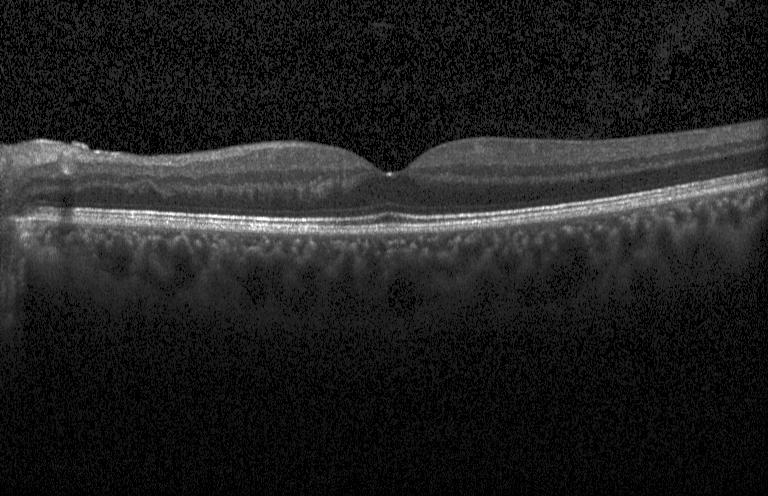 Diagnosis: neither choroidal neovascularization, diabetic macular edema, nor drusen.